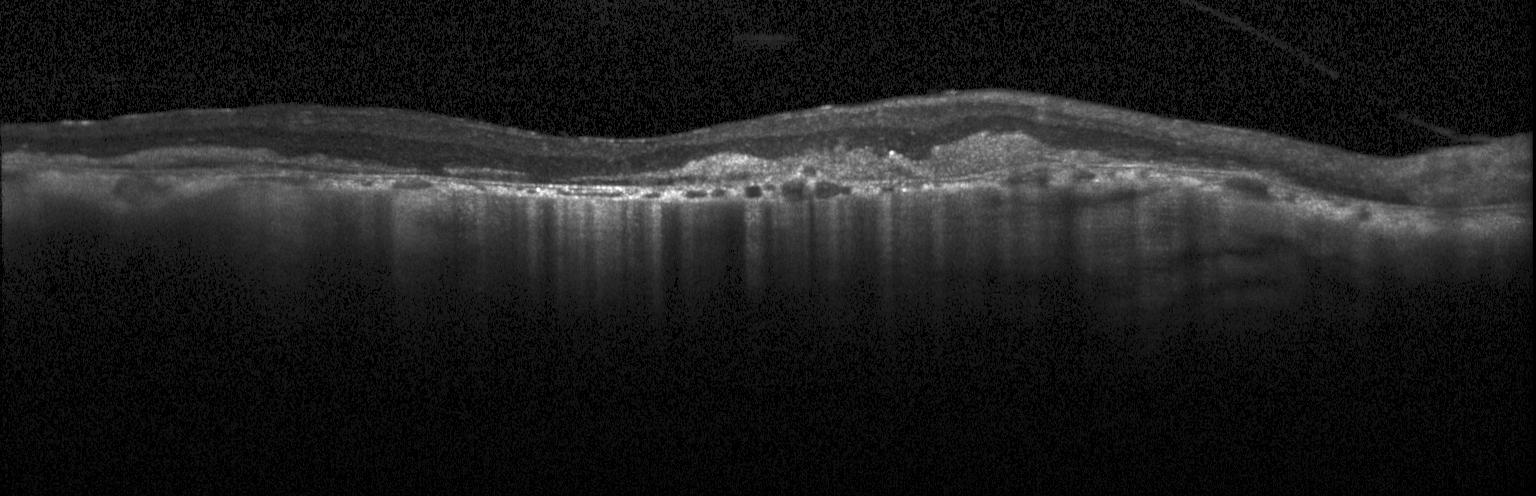
Spectral-domain OCT. Optical coherence tomography scan. Through the macula.
A choroidal neovascular membrane.